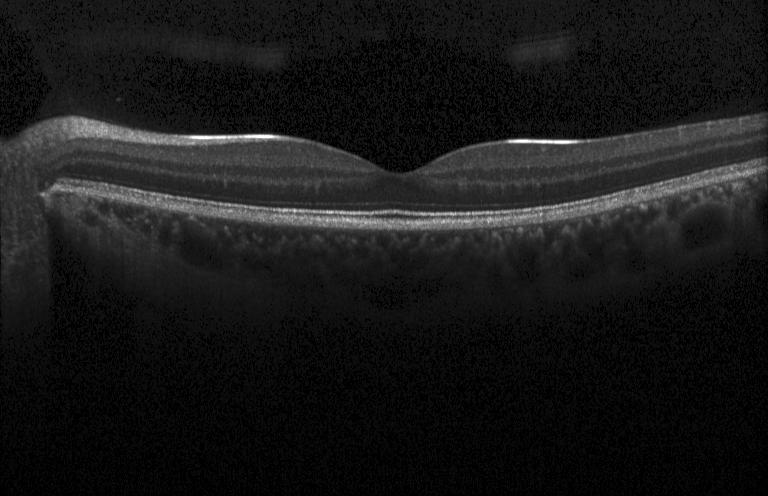 Horizontal scan through the fovea; OCT line scan; Heidelberg Spectralis OCT system; SD-OCT. Finding: neither CNV, DME, nor drusen.